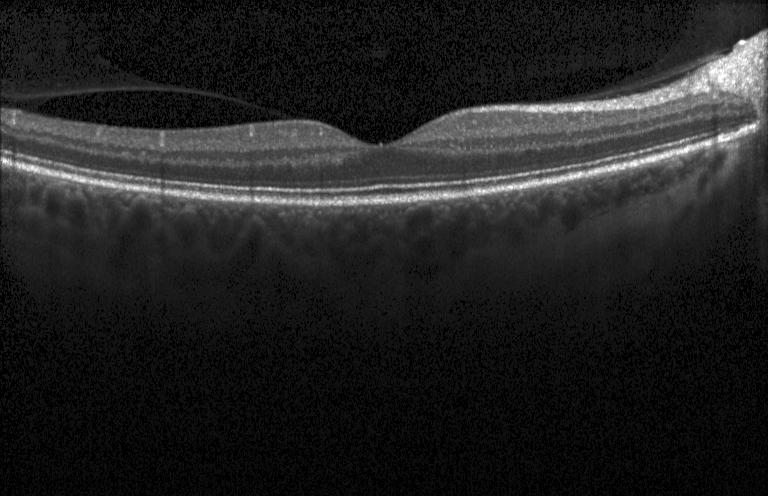 Retinal OCT cross-section — Diagnosis: no choroidal neovascularization, no diabetic macular edema, and no drusen.